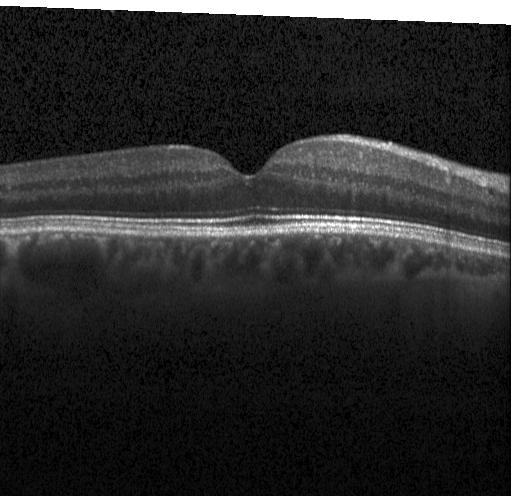

This B-scan demonstrates no CNV, no DME, and no drusen.